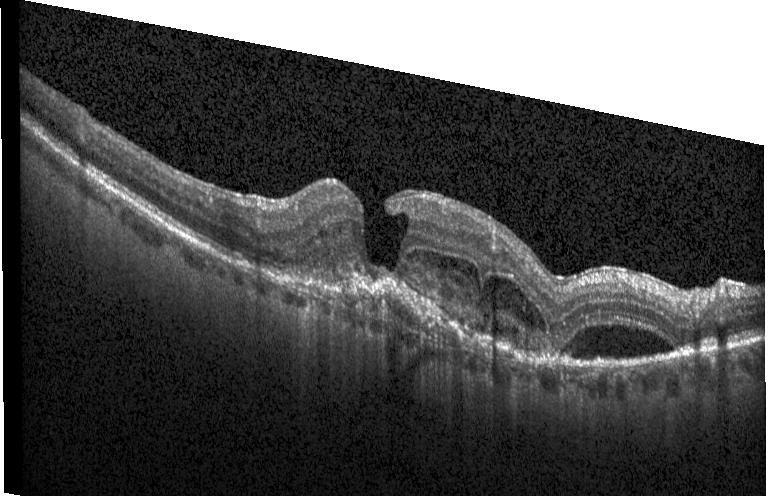

Spectral-domain optical coherence tomography; OCT line scan; fovea-centered — Impression: choroidal neovascularization.